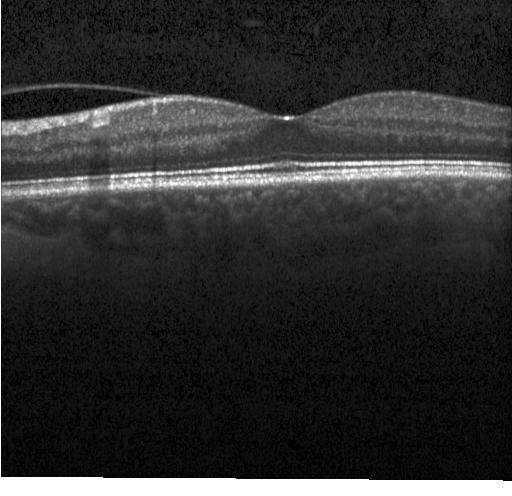

Finding: neither choroidal neovascularization, diabetic macular edema, nor drusen.